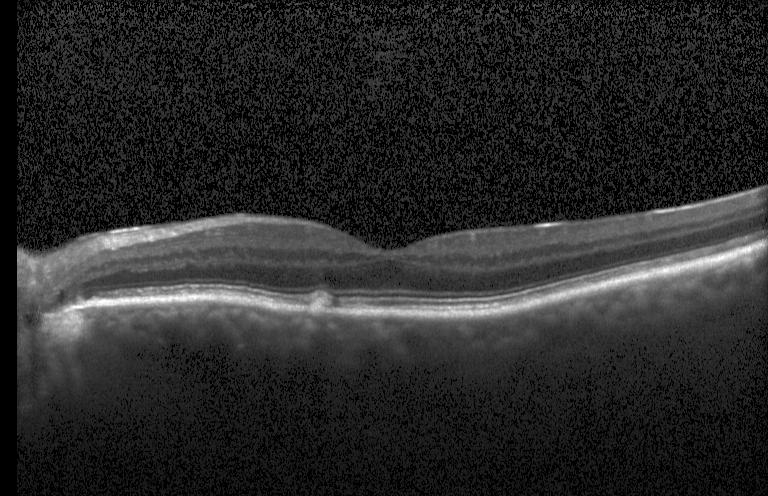 Optical coherence tomography scan. The scan shows sub-RPE drusenoid deposits.